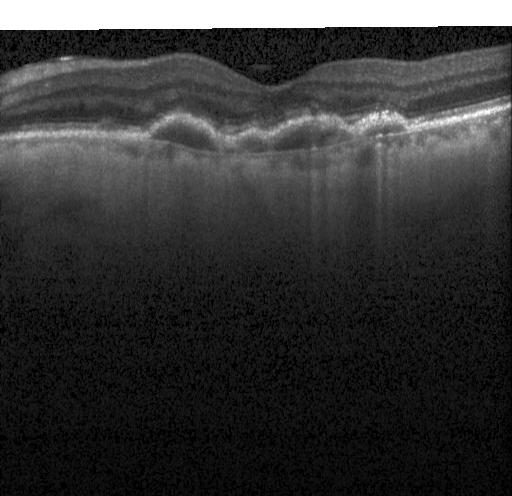 Diagnosis: choroidal neovascularization.